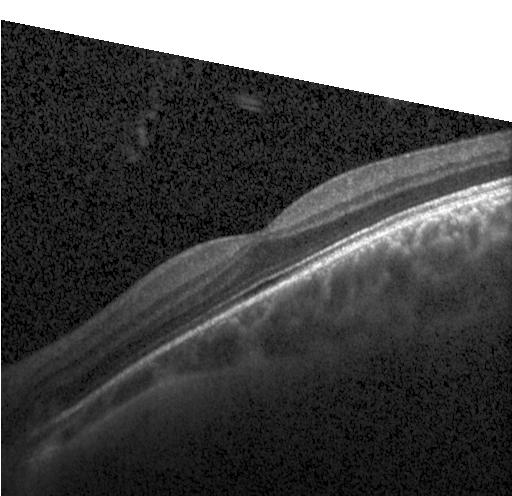
Optical coherence tomography scan, SD-OCT, macular scan, Heidelberg Spectralis OCT system.
Finding: no CNV, no DME, and no drusen.